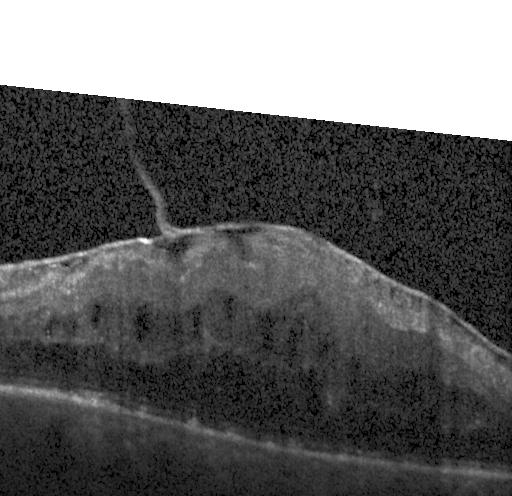 Spectral-domain optical coherence tomography · macular scan · acquired on a Heidelberg Spectralis · OCT line scan. Impression: DME.